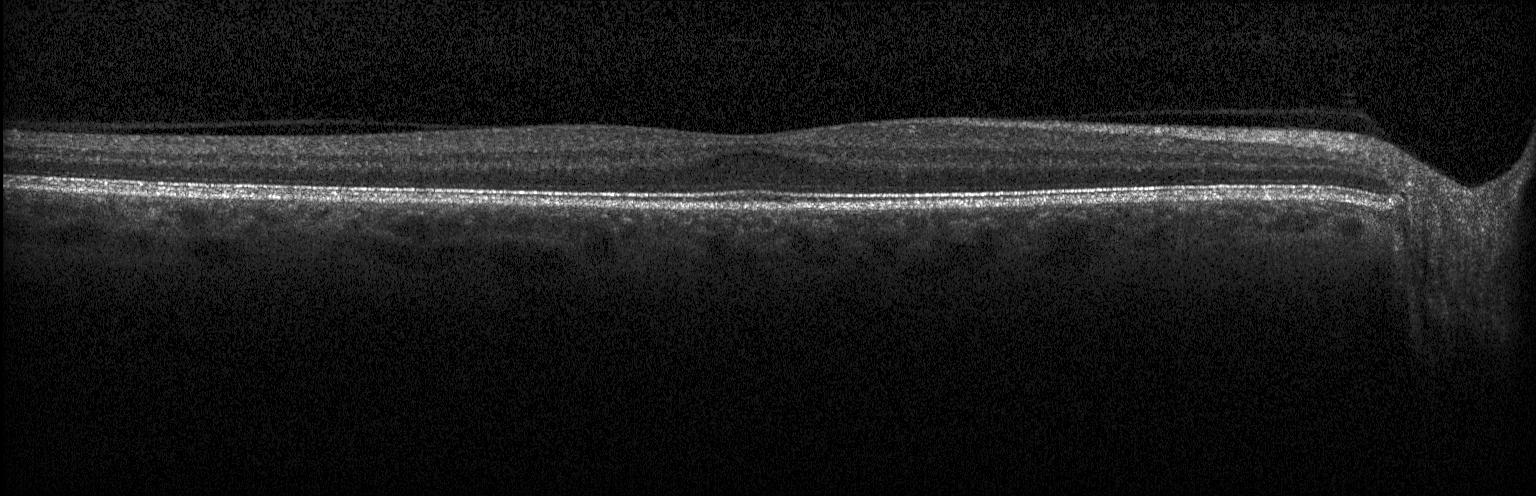
Impression: no choroidal neovascularization, diabetic macular edema, or drusen.